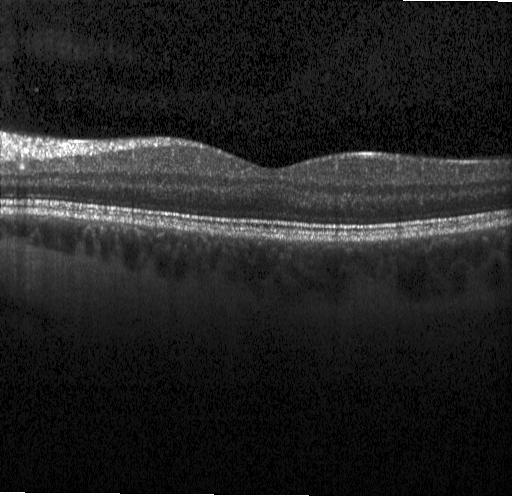
Optical coherence tomography B-scan, macular scan — Impression: no choroidal neovascularization, diabetic macular edema, or drusen.